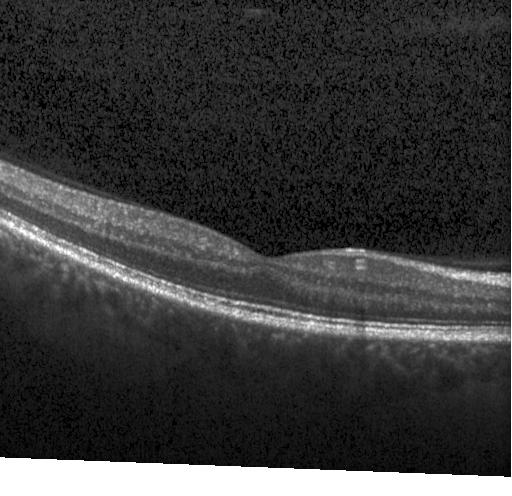

Neither CNV, DME, nor drusen.